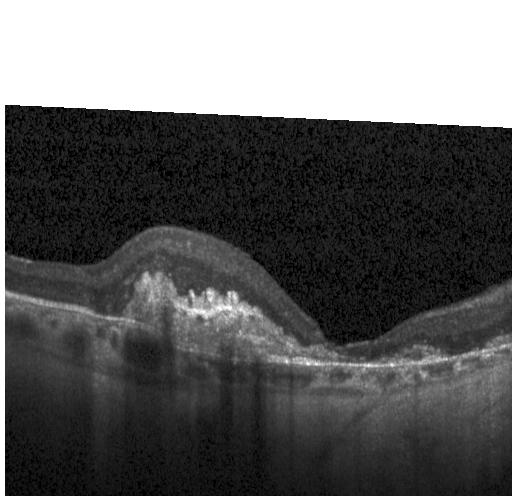
Optical coherence tomography B-scan · SD-OCT · through the macula · Heidelberg Spectralis OCT system
The scan shows a choroidal neovascular membrane.